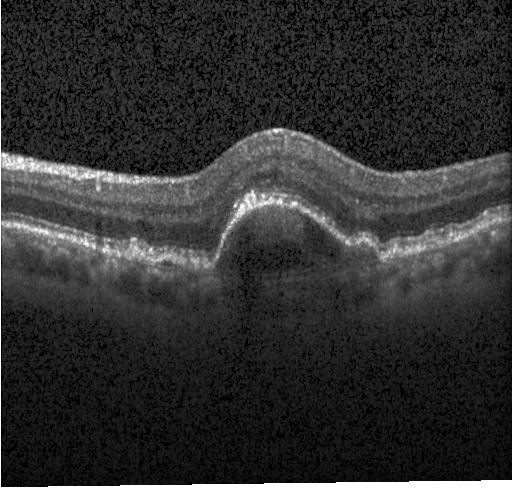

OCT line scan.
Diagnosis: multiple drusen.